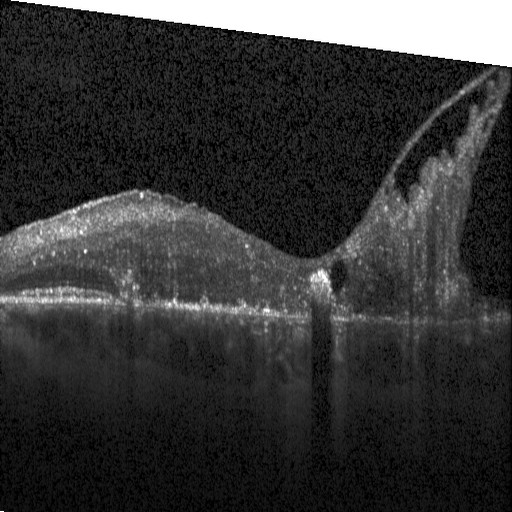 Assessment: diabetic macular edema.